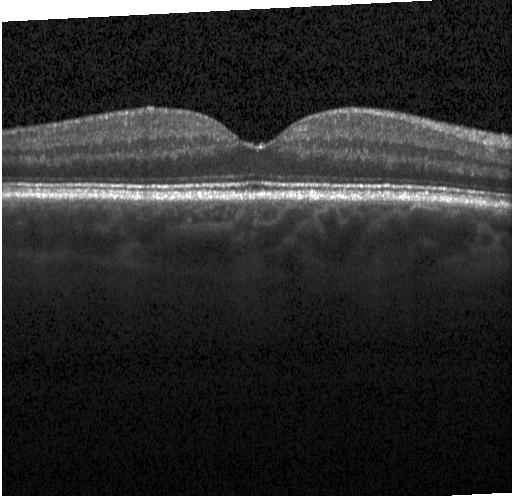 OCT B-scan showing no choroidal neovascularization, no diabetic macular edema, and no drusen.